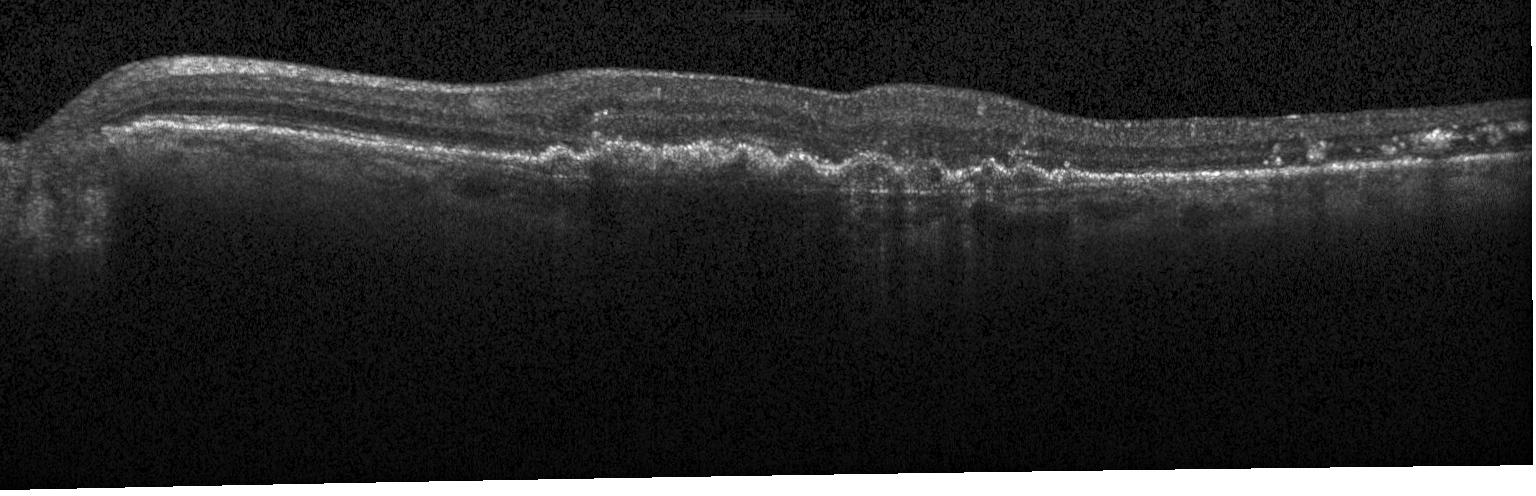

Retinal OCT cross-section showing choroidal neovascularization.